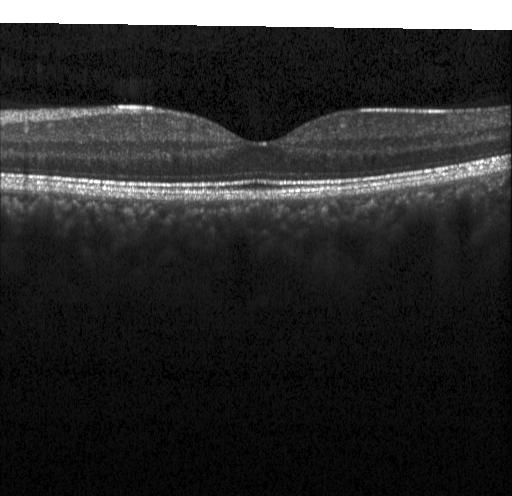

Finding: no CNV, no DME, and no drusen.